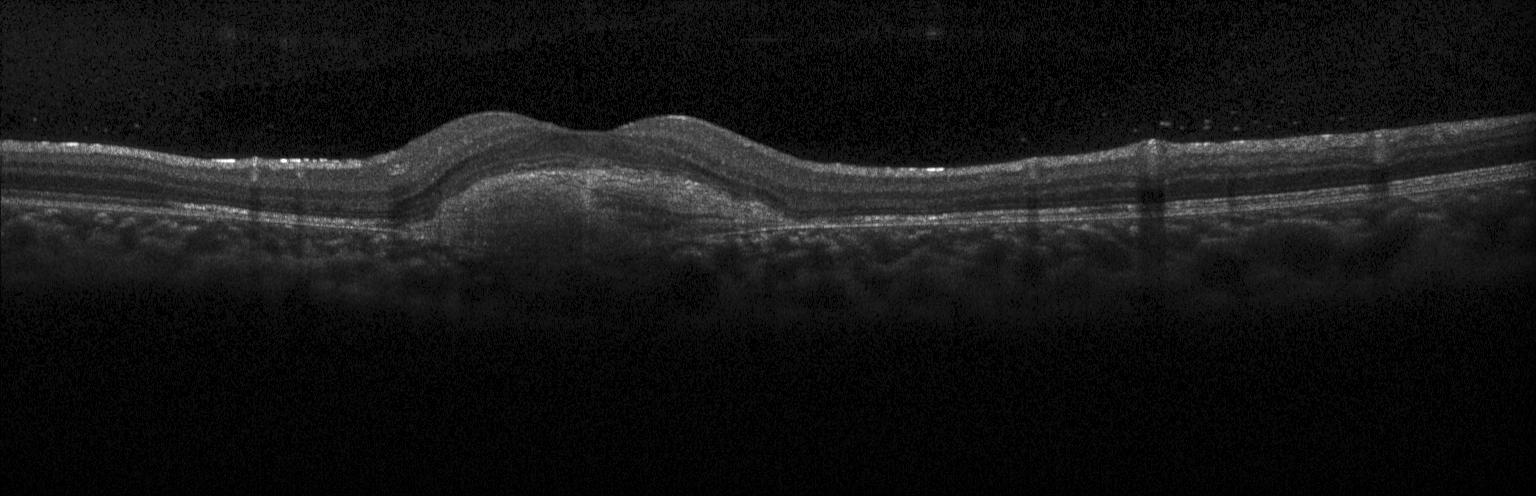

Spectral-domain OCT B-scan: a choroidal neovascular membrane.